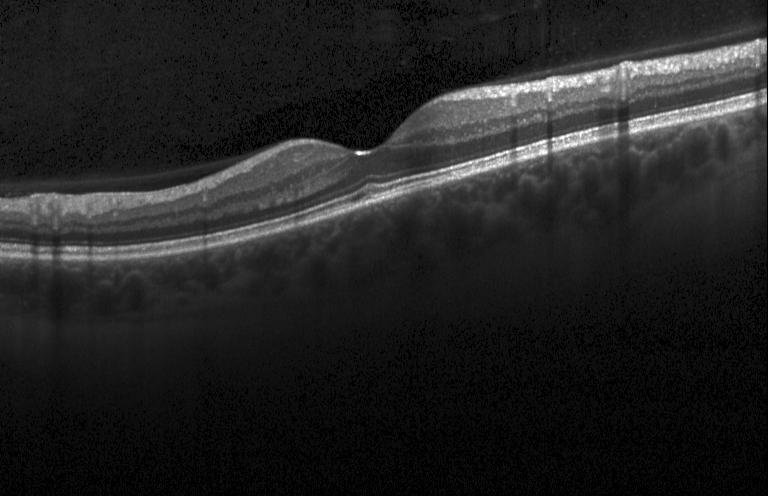

Macular OCT: no choroidal neovascularization, diabetic macular edema, or drusen.